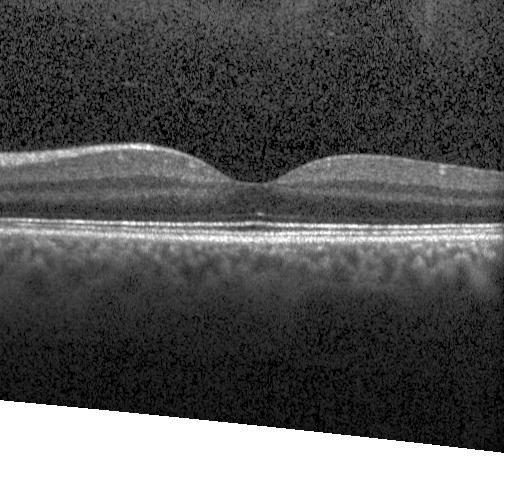
OCT B-scan showing no evidence of CNV, DME, or drusen.